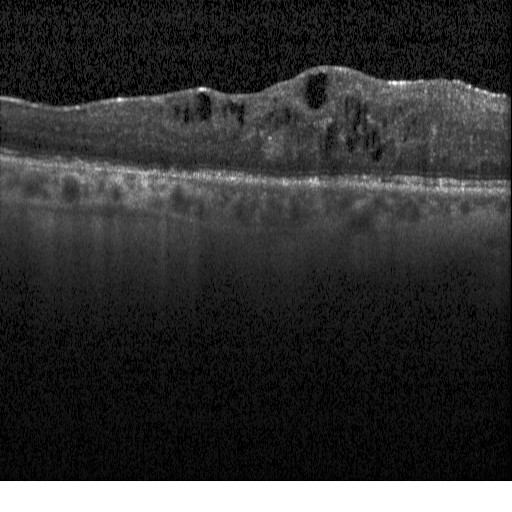

Impression: DME.